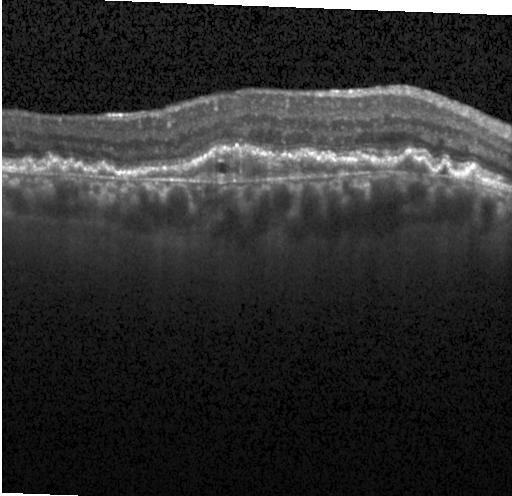 Assessment: a choroidal neovascular membrane.